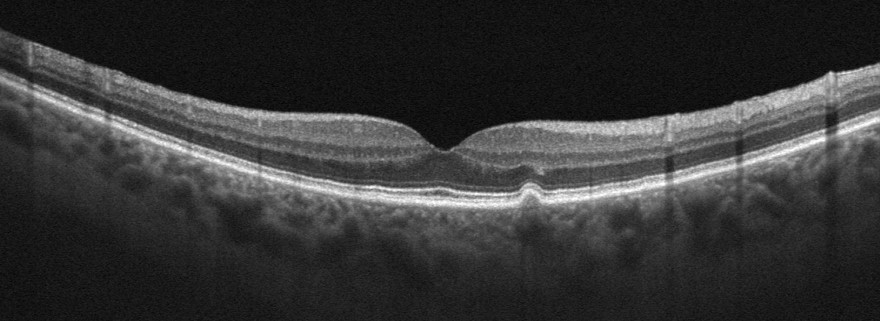

Retinal OCT cross-section · instrument: Optovue Avanti RTVue XR
Impression: AMD.